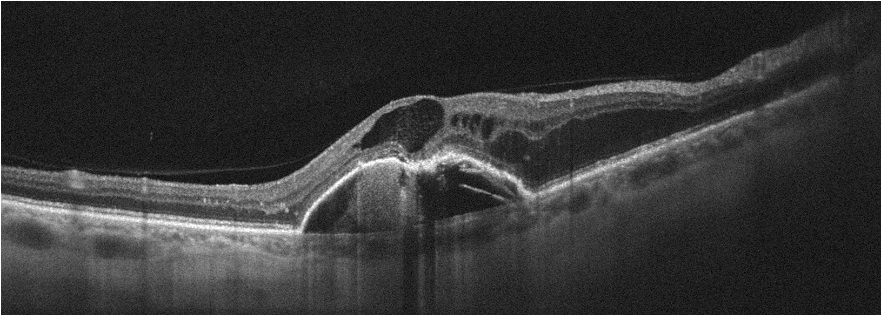 Retinal OCT B-scan · macular scan.
AMD.